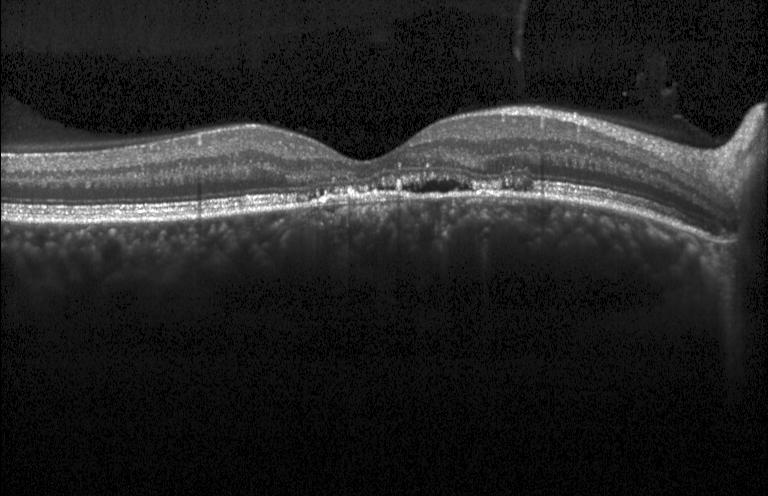
Diagnosis: a choroidal neovascular membrane.